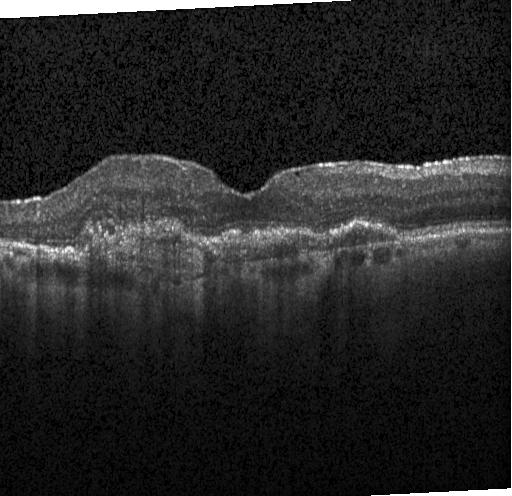
Optical coherence tomography scan — Finding: choroidal neovascularization (CNV).